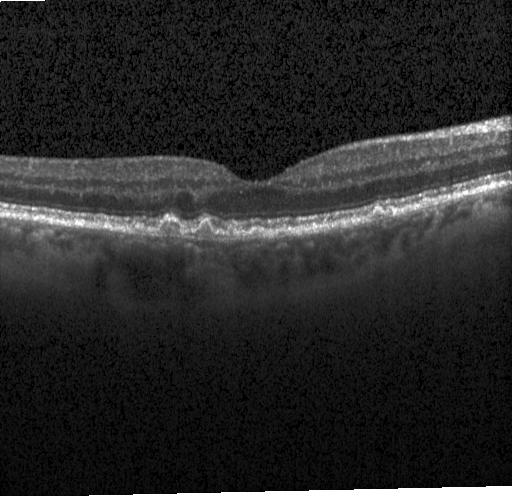
Acquired on a Heidelberg Spectralis · horizontal scan through the fovea · optical coherence tomography B-scan · spectral-domain optical coherence tomography — Diagnosis: sub-RPE drusenoid deposits.